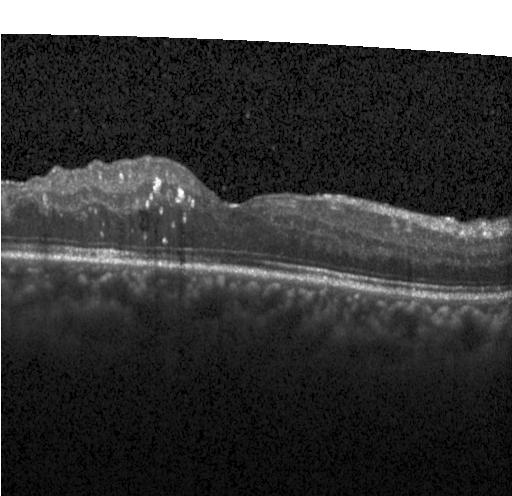

Instrument: Heidelberg Spectralis. Spectral-domain OCT. OCT line scan
OCT finding: DME.